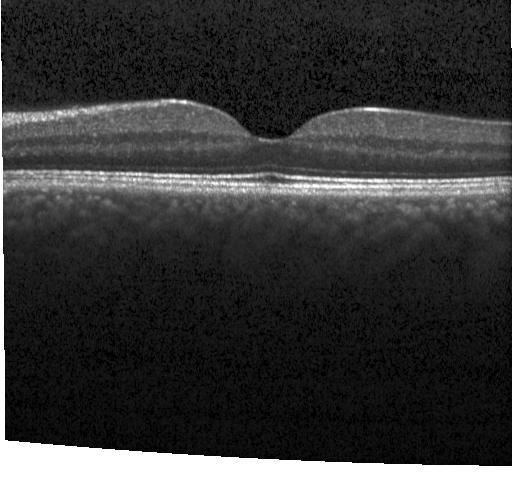 Finding: no choroidal neovascularization, diabetic macular edema, or drusen.